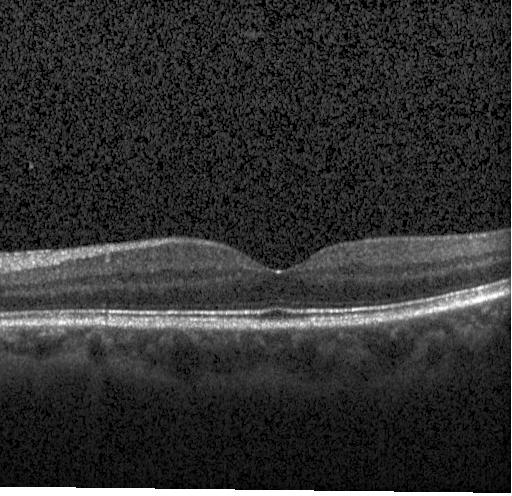

Spectral-domain optical coherence tomography · retinal OCT B-scan
Finding: no choroidal neovascularization, no diabetic macular edema, and no drusen.